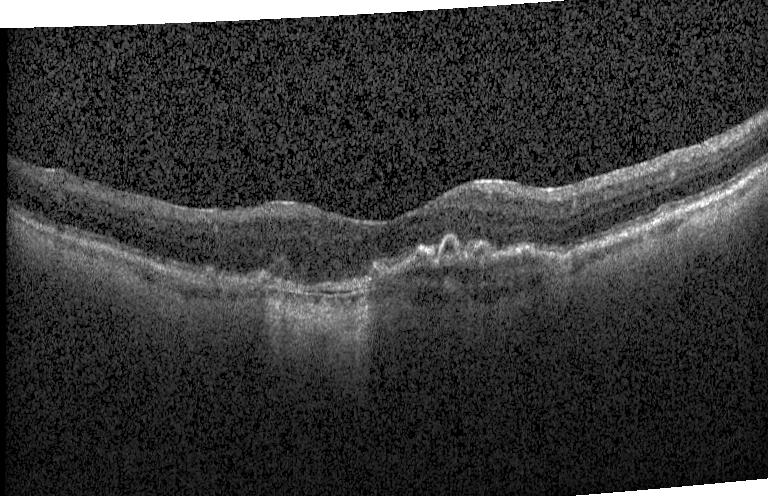
Retinal OCT cross-section showing CNV.